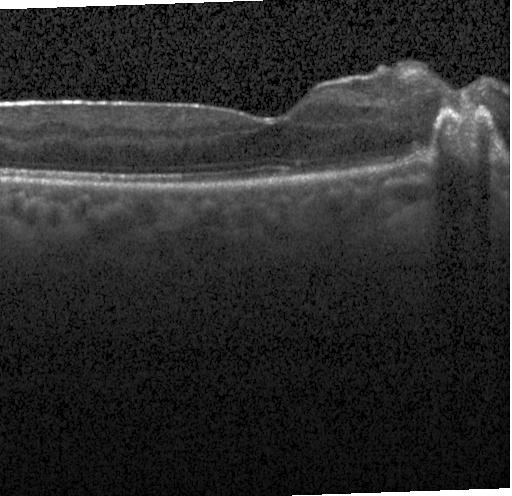

Retinal OCT cross-section showing CNV.